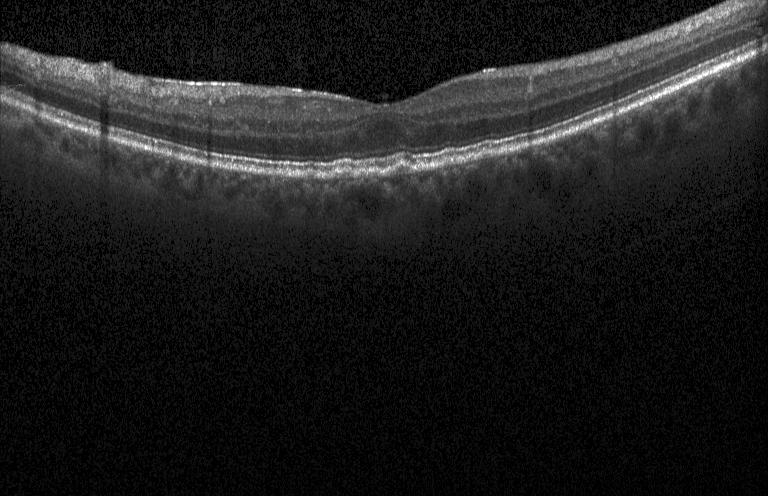 Spectral-domain OCT, macular scan, optical coherence tomography B-scan — OCT finding: sub-RPE drusenoid deposits.